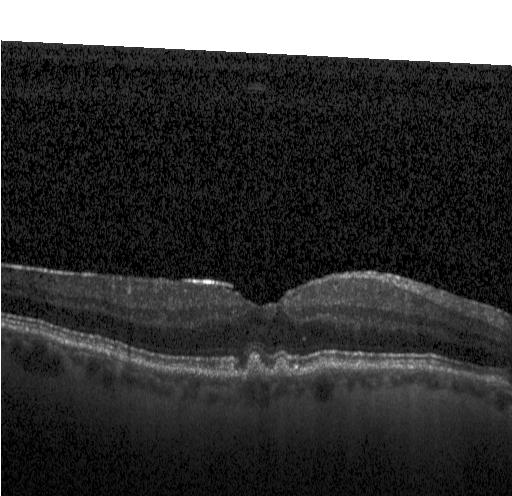
Retinal OCT cross-section · spectral-domain optical coherence tomography · macular scan · Heidelberg Spectralis OCT system — OCT finding: sub-RPE drusenoid deposits.